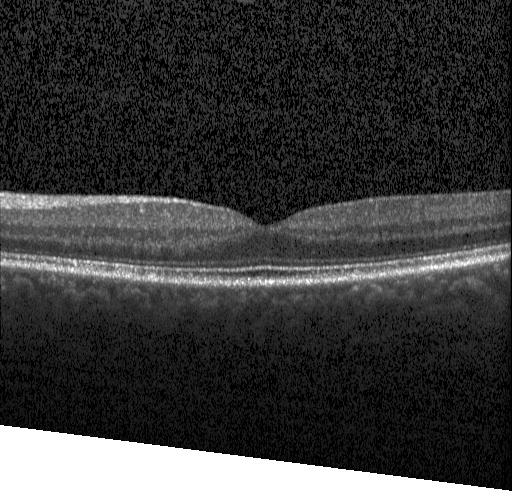 Optical coherence tomography B-scan.
The scan shows no choroidal neovascularization, diabetic macular edema, or drusen.